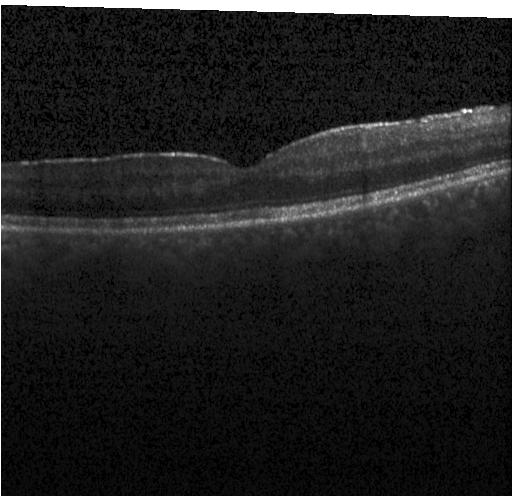
Acquired on a Heidelberg Spectralis. Optical coherence tomography scan. SD-OCT.
Dx: no choroidal neovascularization, no diabetic macular edema, and no drusen.